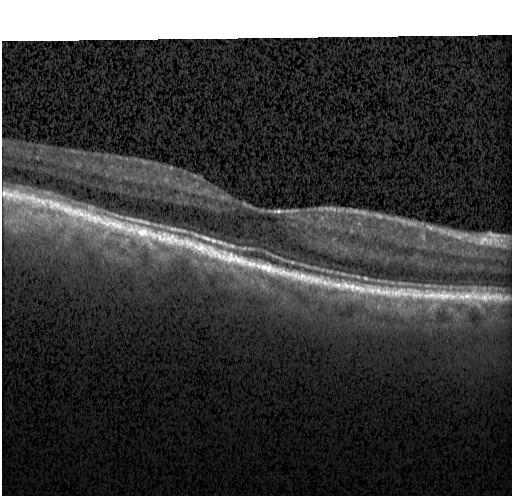
Impression: no choroidal neovascularization, no diabetic macular edema, and no drusen.